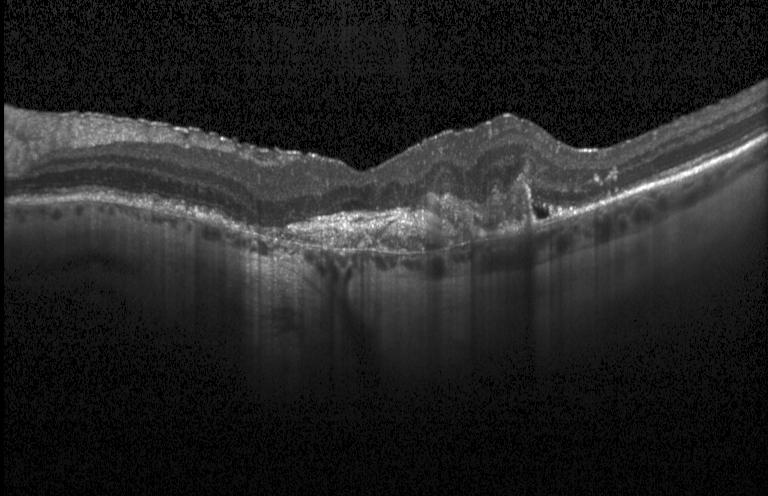

Retinal OCT B-scan
Diagnosis: a choroidal neovascular membrane.